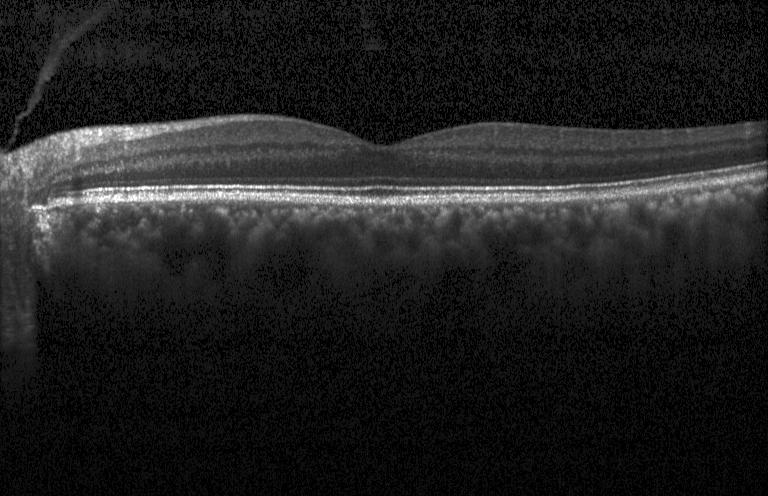

Instrument: Heidelberg Spectralis; through the macula; spectral-domain OCT; optical coherence tomography scan. Finding: neither CNV, DME, nor drusen.